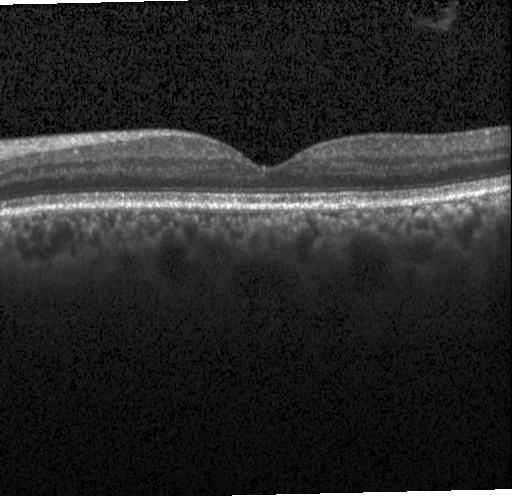
Retinal OCT cross-section
No choroidal neovascularization, diabetic macular edema, or drusen.